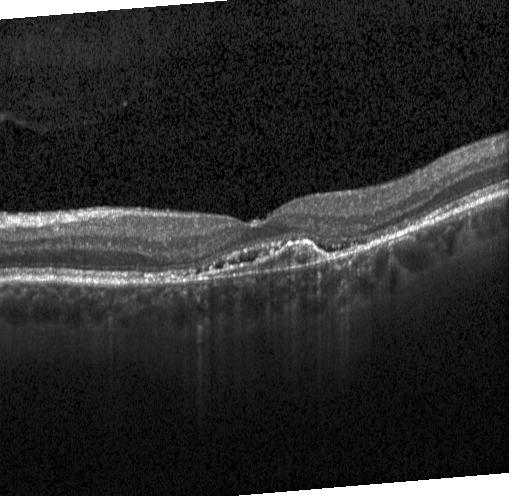 Assessment: CNV.